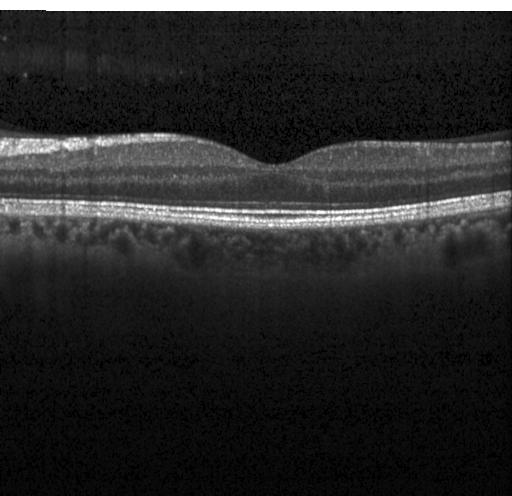
Acquired on a Heidelberg Spectralis. Optical coherence tomography B-scan.
Finding: no choroidal neovascularization, no diabetic macular edema, and no drusen.